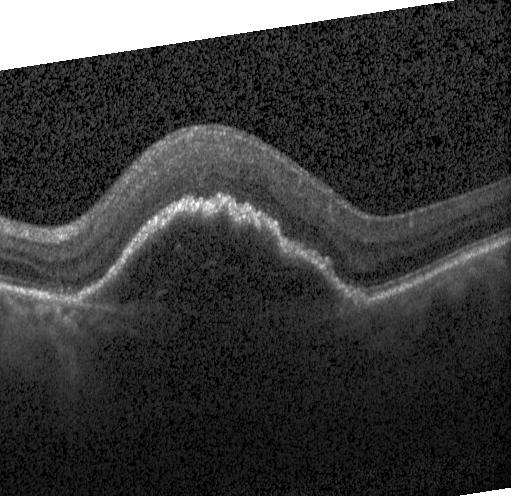

OCT finding: choroidal neovascularization.